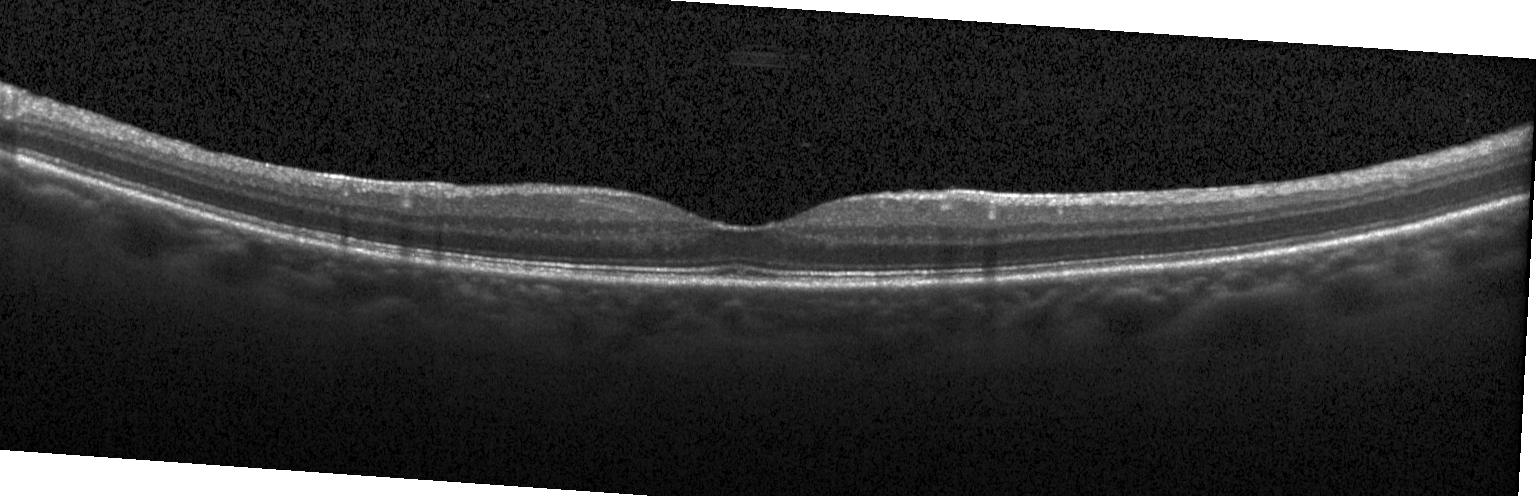
No evidence of choroidal neovascularization, diabetic macular edema, or drusen.